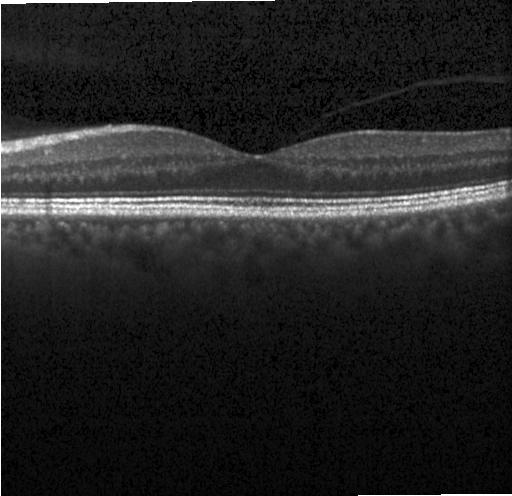 Optical coherence tomography B-scan, Heidelberg Spectralis — OCT finding: no evidence of choroidal neovascularization, diabetic macular edema, or drusen.